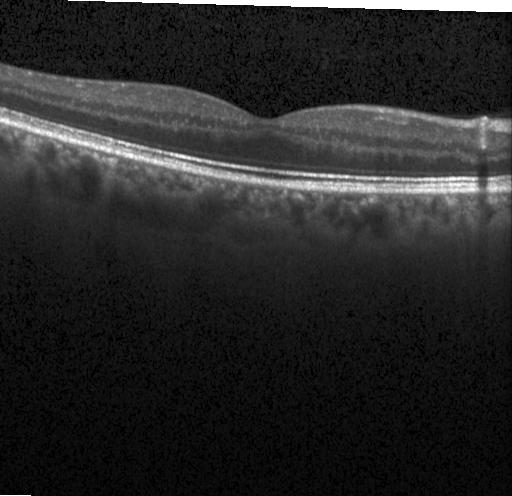 Dx: neither choroidal neovascularization, diabetic macular edema, nor drusen.